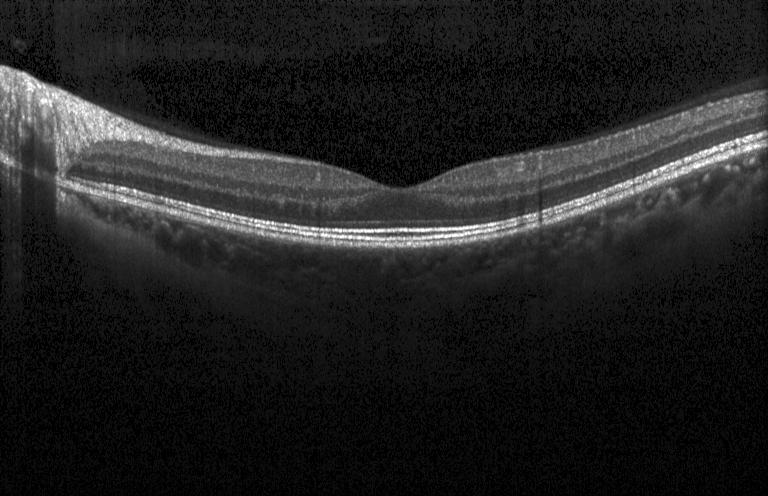

Retinal OCT cross-section. Spectral-domain OCT. Heidelberg Spectralis OCT system. Fovea-centered. The scan shows no evidence of choroidal neovascularization, diabetic macular edema, or drusen.